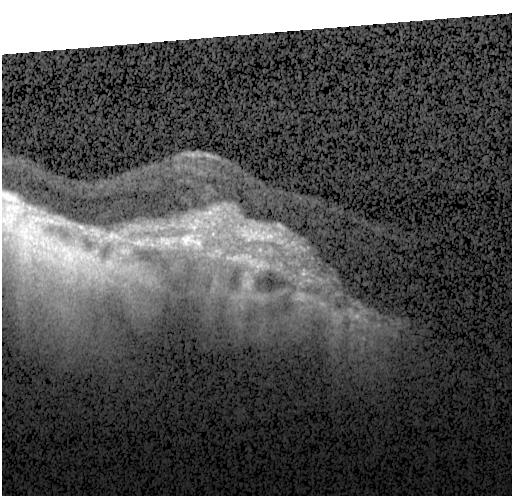
OCT B-scan
Finding: choroidal neovascularization (CNV).